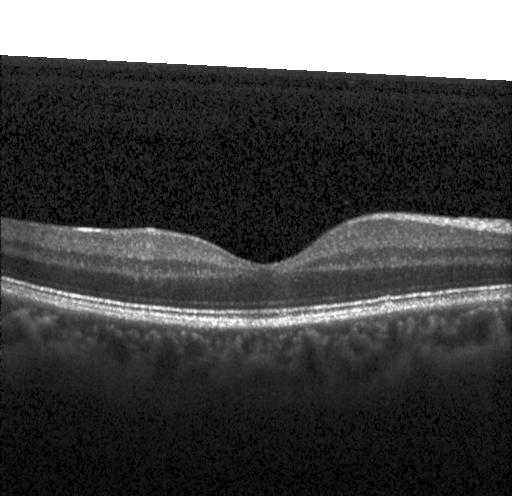 Spectral-domain optical coherence tomography. Retinal OCT cross-section.
Impression: no CNV, DME, or drusen.